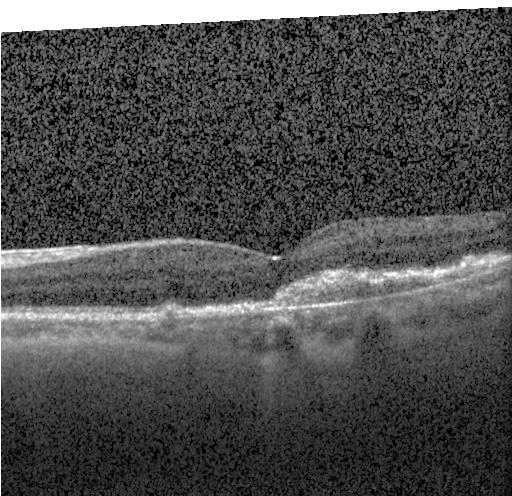 Macular OCT demonstrating choroidal neovascularization.